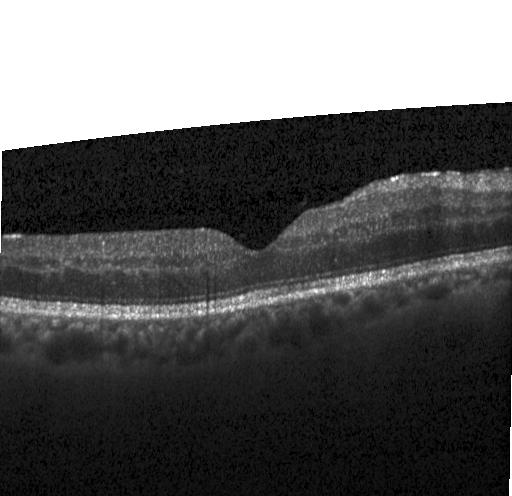 Retinal OCT B-scan · macular scan · Heidelberg Spectralis OCT system.
This B-scan demonstrates no evidence of choroidal neovascularization, diabetic macular edema, or drusen.